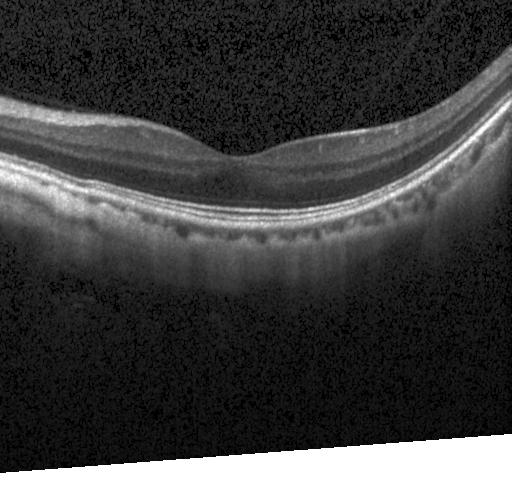 OCT scan showing no choroidal neovascularization, diabetic macular edema, or drusen.